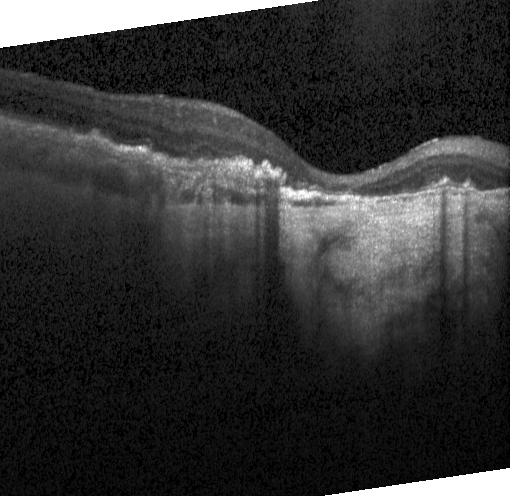 Retinal OCT B-scan; fovea-centered; Heidelberg Spectralis. Assessment: CNV.